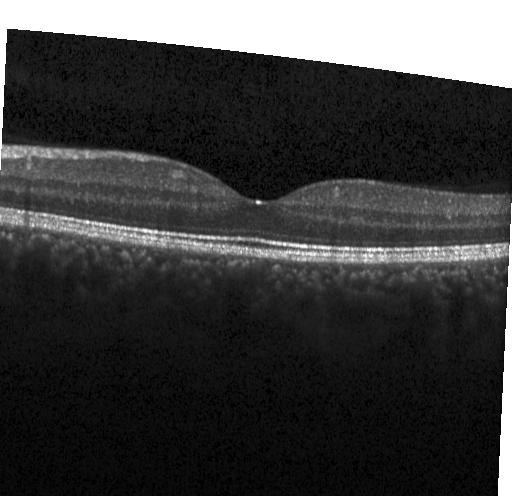

Retinal OCT cross-section. Heidelberg Spectralis. Fovea-centered. Finding: neither choroidal neovascularization, diabetic macular edema, nor drusen.